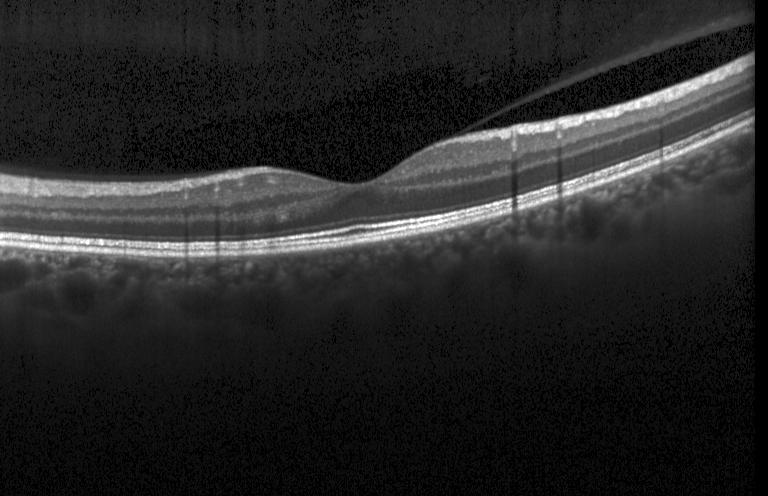 Centered on the fovea; optical coherence tomography scan; spectral-domain OCT; acquired on a Heidelberg Spectralis — OCT finding: no evidence of choroidal neovascularization, diabetic macular edema, or drusen.